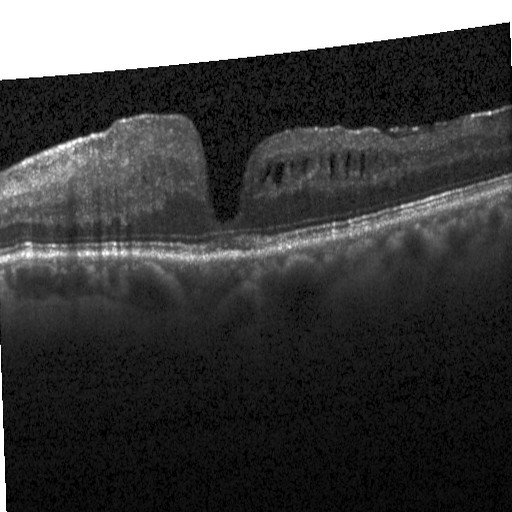 Finding: diabetic macular edema (DME).